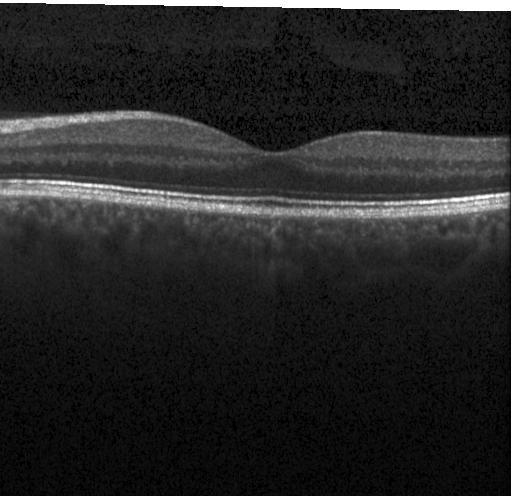
OCT B-scan. Instrument: Heidelberg Spectralis. Fovea-centered. Finding: neither choroidal neovascularization, diabetic macular edema, nor drusen.